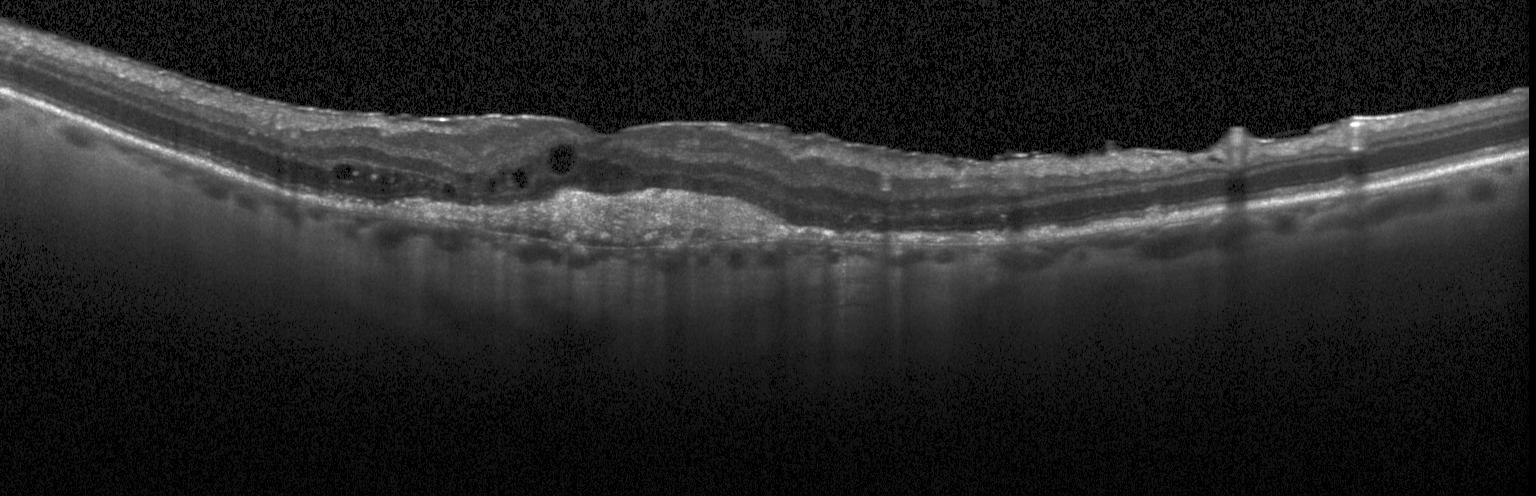
Optical coherence tomography scan; Heidelberg Spectralis; fovea-centered. Diagnosis: choroidal neovascularization (CNV).